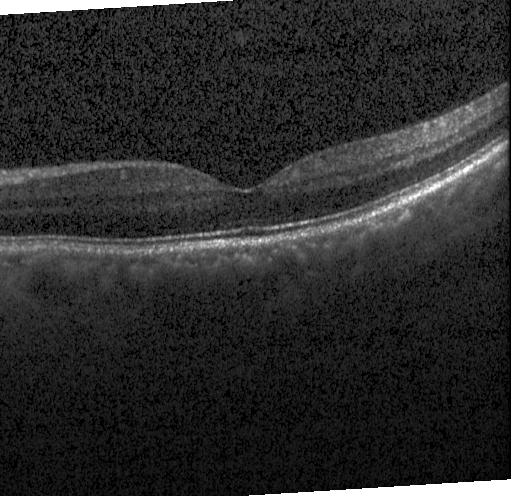
Spectral-domain OCT B-scan: neither choroidal neovascularization, diabetic macular edema, nor drusen.